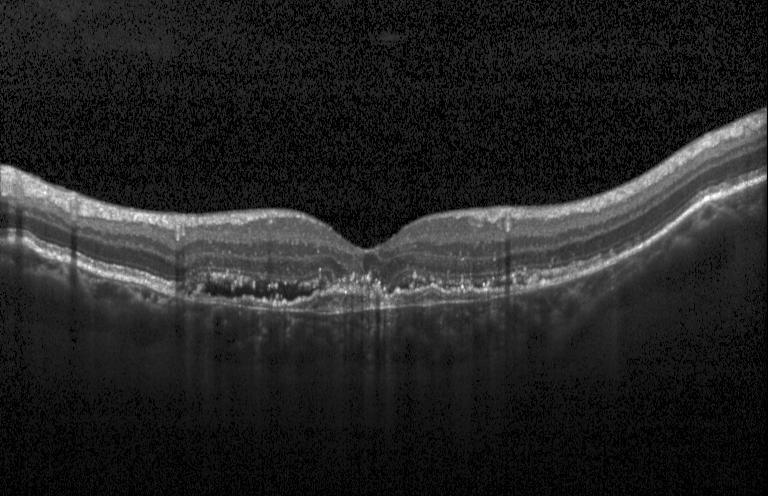
Instrument: Heidelberg Spectralis, retinal OCT cross-section — Impression: choroidal neovascularization (CNV).